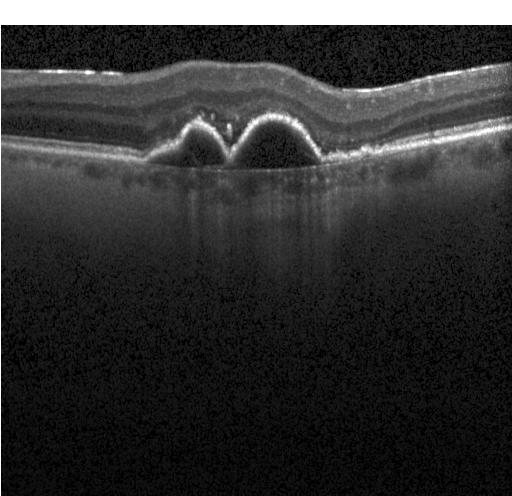
Instrument: Heidelberg Spectralis; OCT B-scan — This B-scan demonstrates a choroidal neovascular membrane.